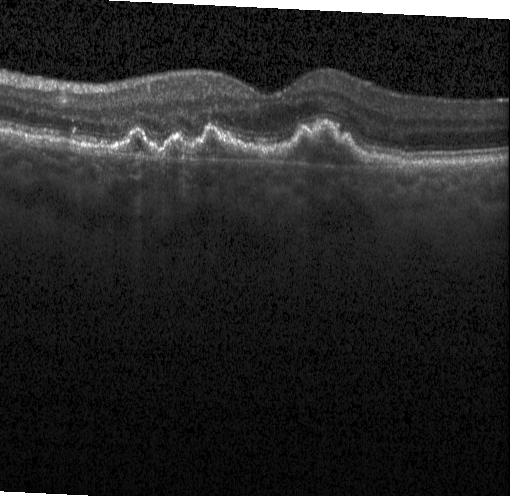 Retinal OCT cross-section.
Diagnosis: choroidal neovascularization.